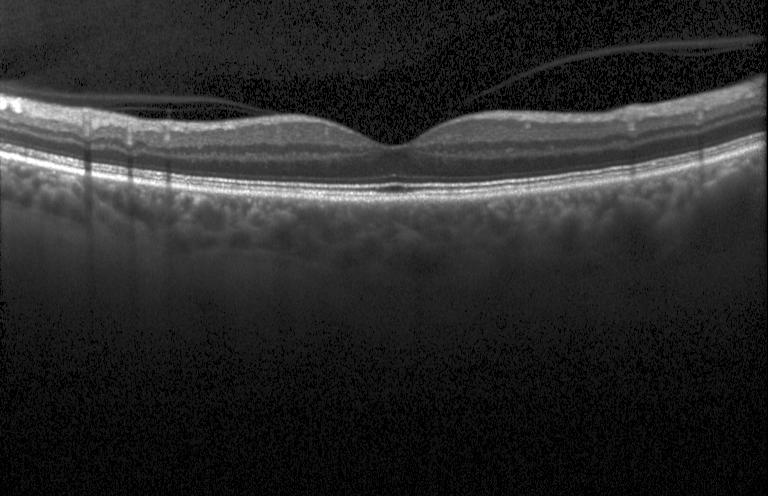 Dx: neither choroidal neovascularization, diabetic macular edema, nor drusen.